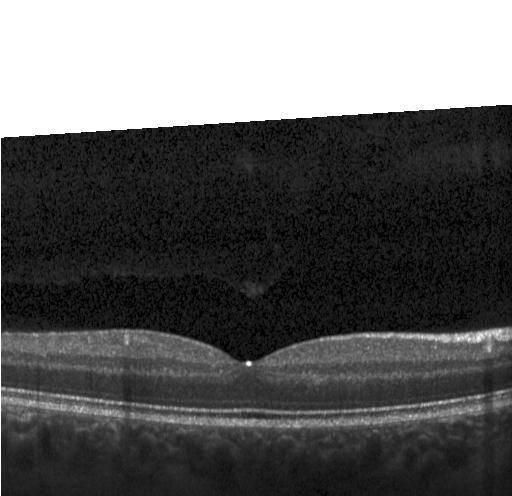 Instrument: Heidelberg Spectralis · retinal OCT cross-section
Dx: no choroidal neovascularization, no diabetic macular edema, and no drusen.